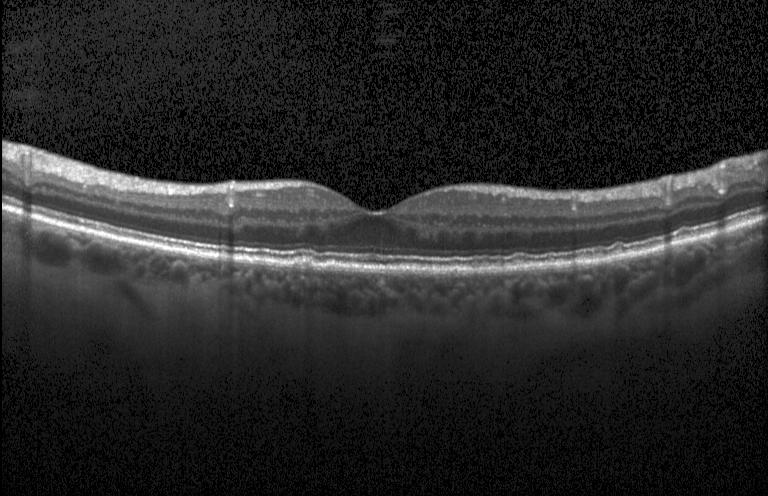 Heidelberg Spectralis OCT system, retinal OCT cross-section. This B-scan demonstrates multiple drusen.